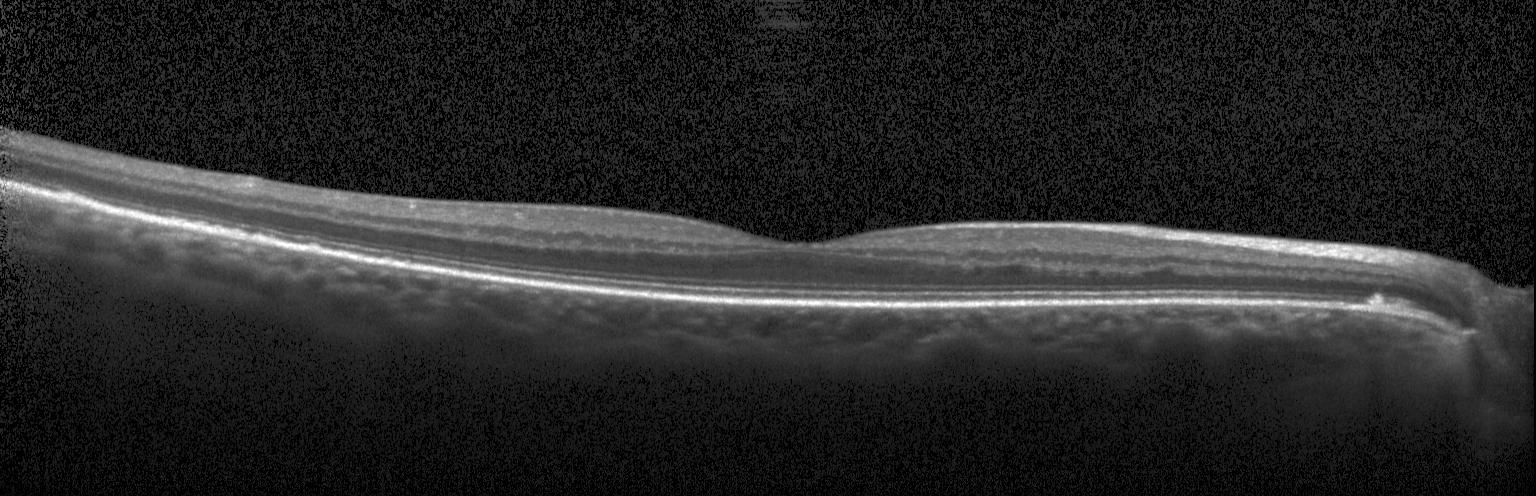
OCT scan showing no choroidal neovascularization, no diabetic macular edema, and no drusen.